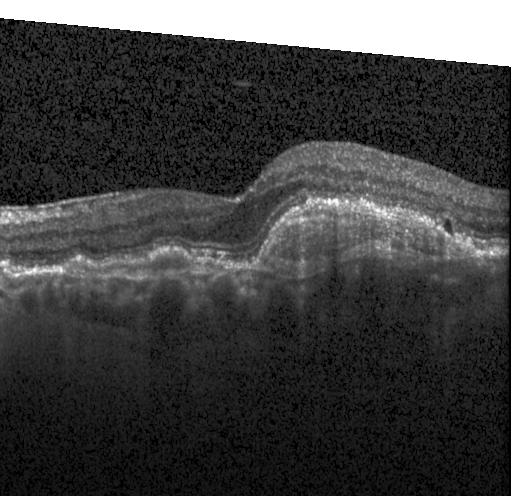 Spectral-domain OCT B-scan: a choroidal neovascular membrane.